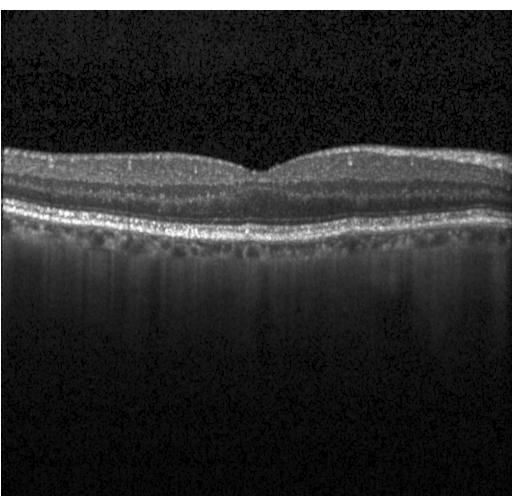

Retinal OCT cross-section showing no evidence of choroidal neovascularization, diabetic macular edema, or drusen.